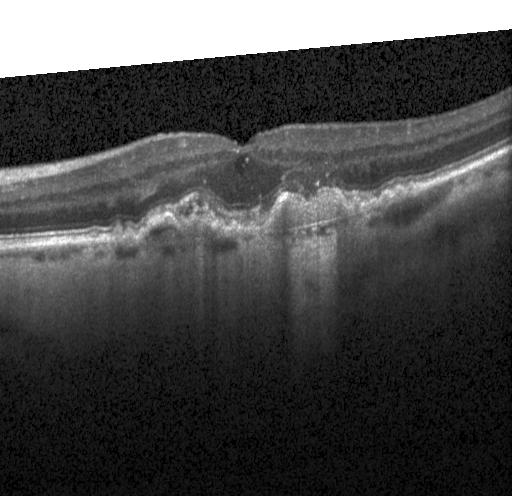 Spectral-domain OCT B-scan: a choroidal neovascular membrane.